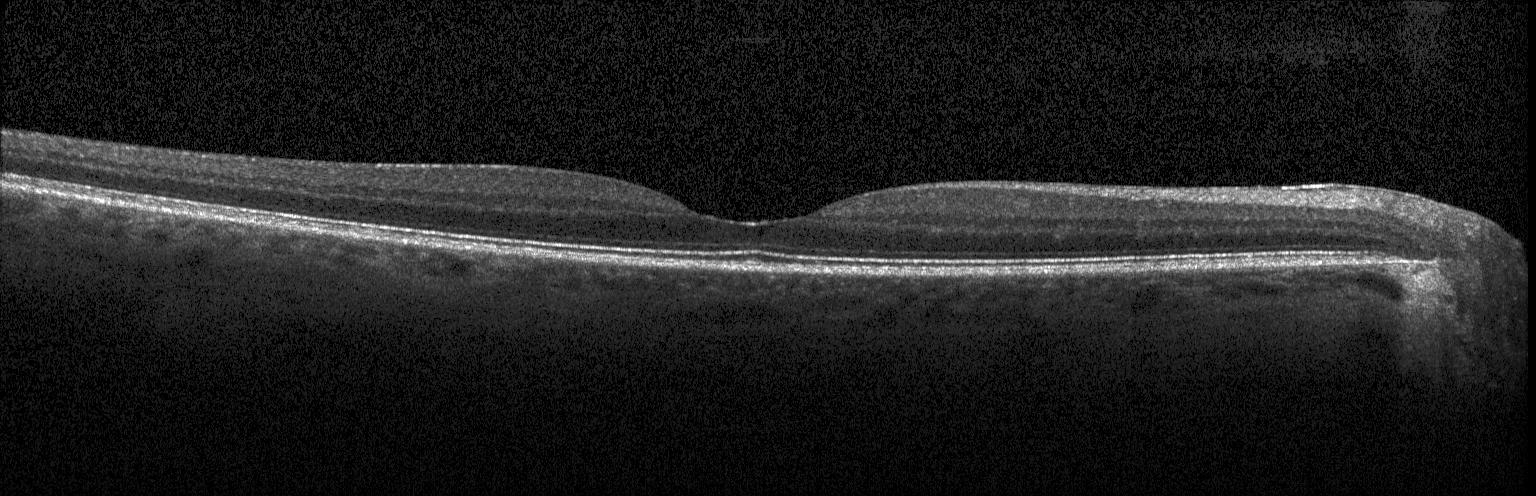
Dx: neither choroidal neovascularization, diabetic macular edema, nor drusen.